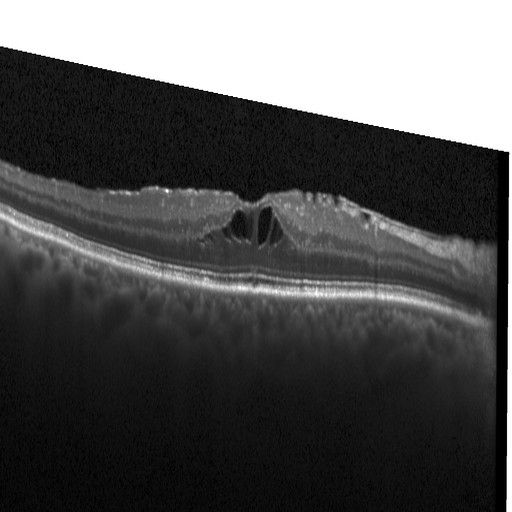 Impression: diabetic macular edema.